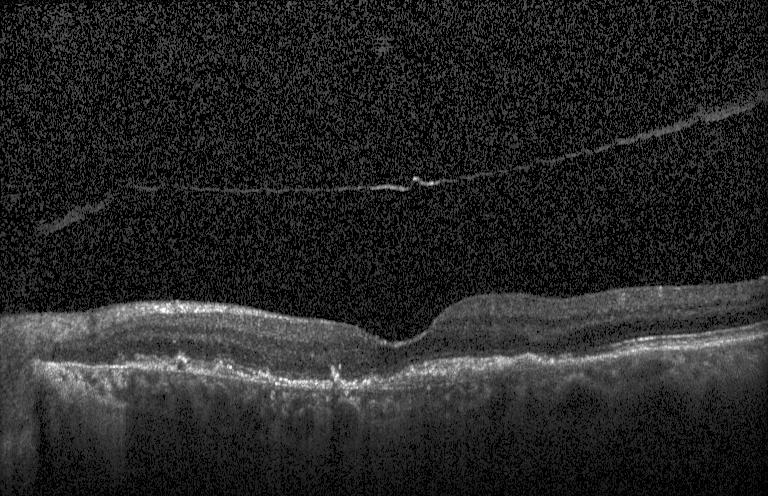 Heidelberg Spectralis · OCT B-scan. This B-scan demonstrates a choroidal neovascular membrane.